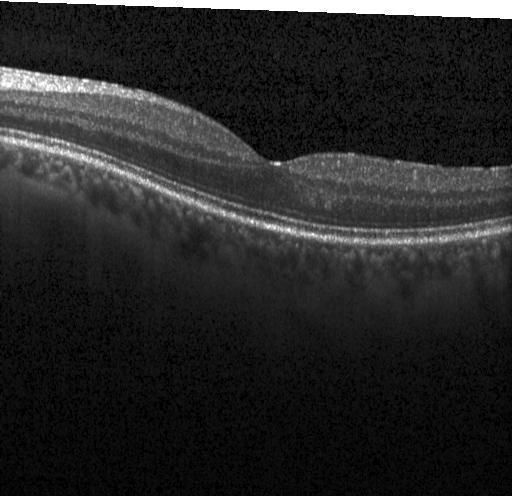 Fovea-centered. Optical coherence tomography B-scan. Diagnosis: no evidence of choroidal neovascularization, diabetic macular edema, or drusen.